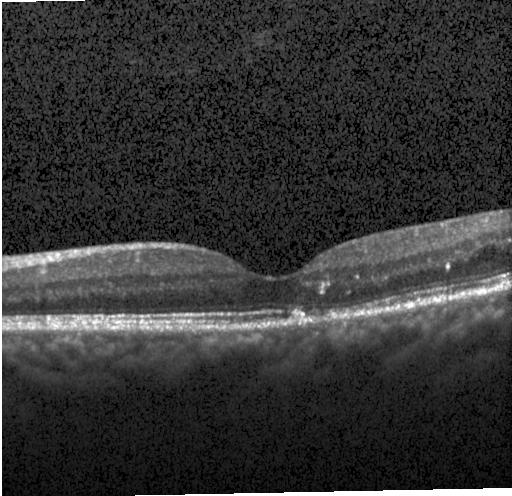

OCT line scan
Diabetic macular edema (DME).